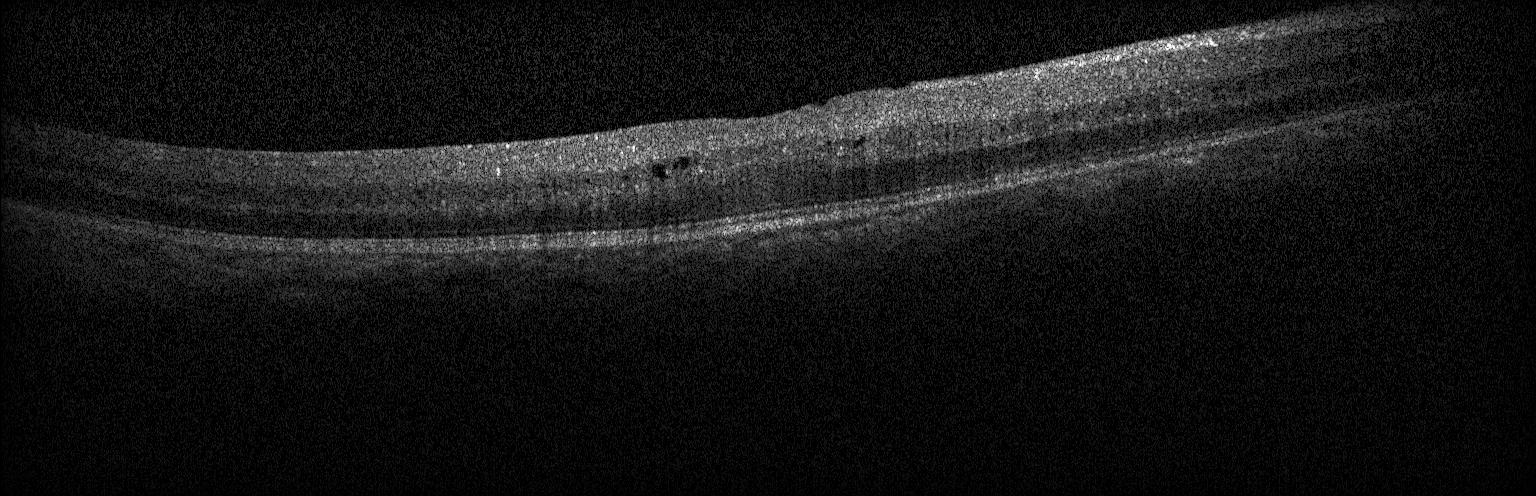

OCT line scan. Impression: diabetic macular edema.